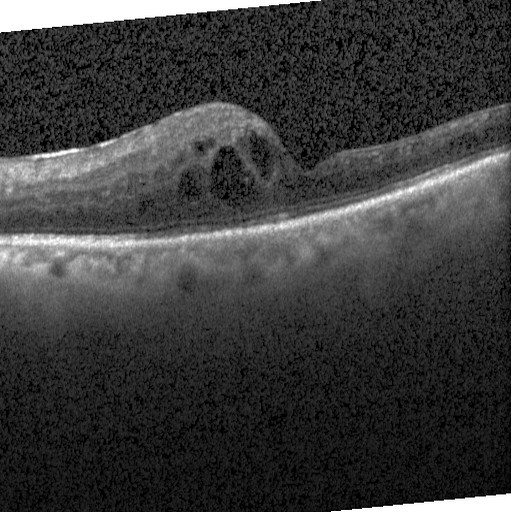
Spectral-domain OCT B-scan: DME.